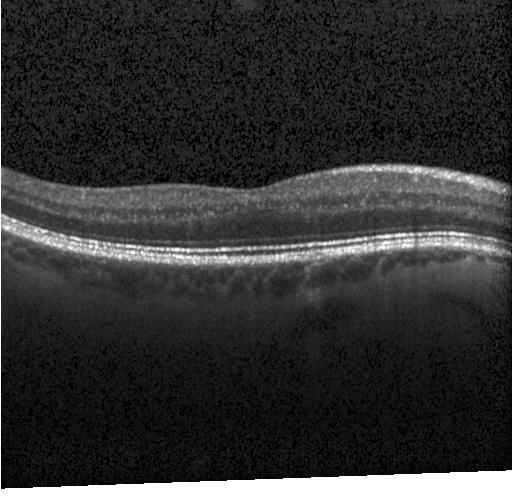
Horizontal scan through the fovea · optical coherence tomography scan · acquired on a Heidelberg Spectralis. Dx: no choroidal neovascularization, diabetic macular edema, or drusen.